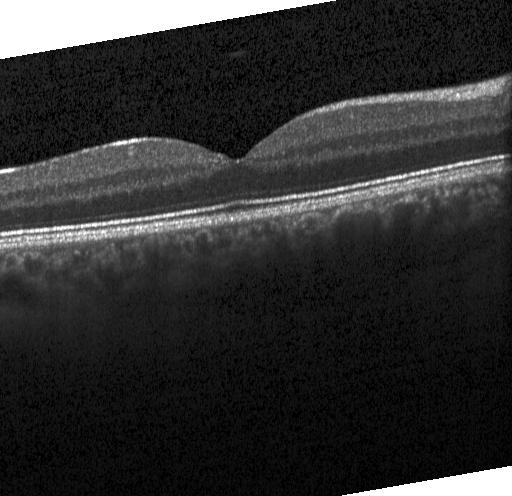

Horizontal scan through the fovea, SD-OCT, OCT B-scan, Heidelberg Spectralis OCT system. Neither choroidal neovascularization, diabetic macular edema, nor drusen.